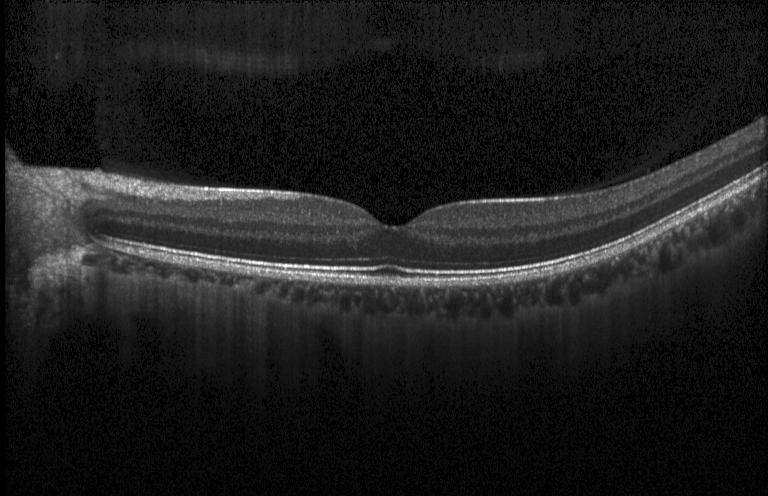 OCT B-scan. Heidelberg Spectralis OCT system. Through the macula.
Impression: no CNV, DME, or drusen.